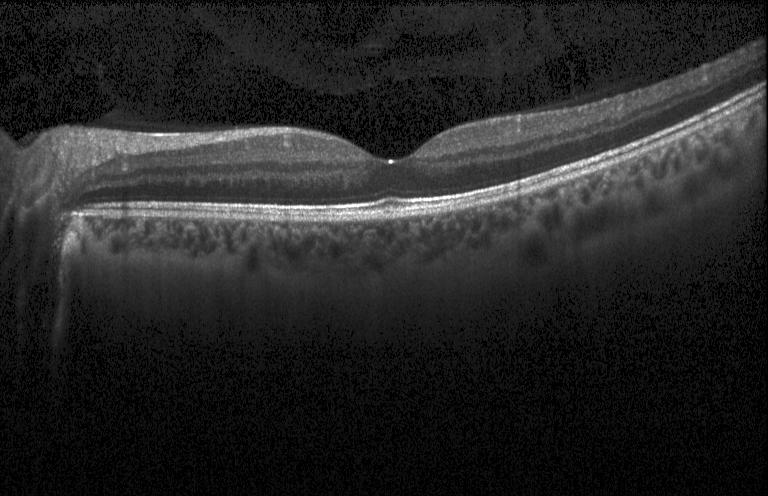 Centered on the fovea, OCT line scan. Dx: no choroidal neovascularization, no diabetic macular edema, and no drusen.